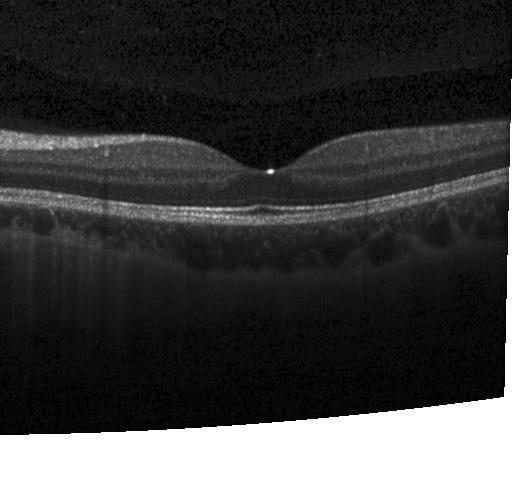
OCT B-scan; fovea-centered; spectral-domain OCT; Heidelberg Spectralis — This B-scan demonstrates neither choroidal neovascularization, diabetic macular edema, nor drusen.